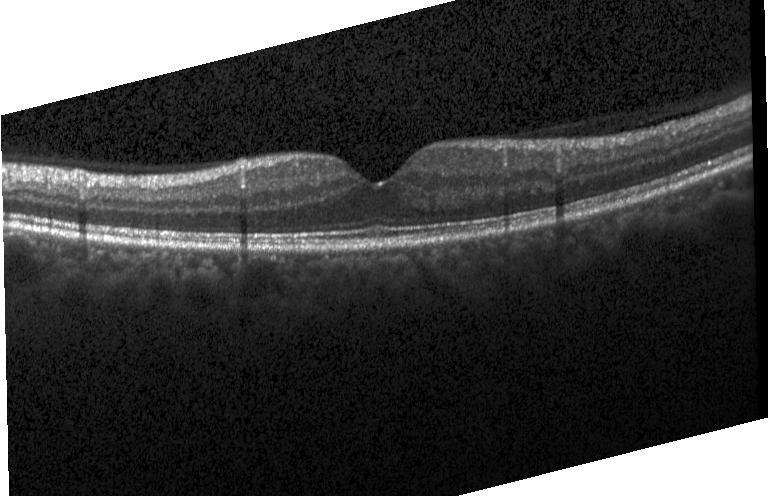 Heidelberg Spectralis OCT system, macular scan, spectral-domain OCT, retinal OCT cross-section.
OCT finding: no CNV, DME, or drusen.